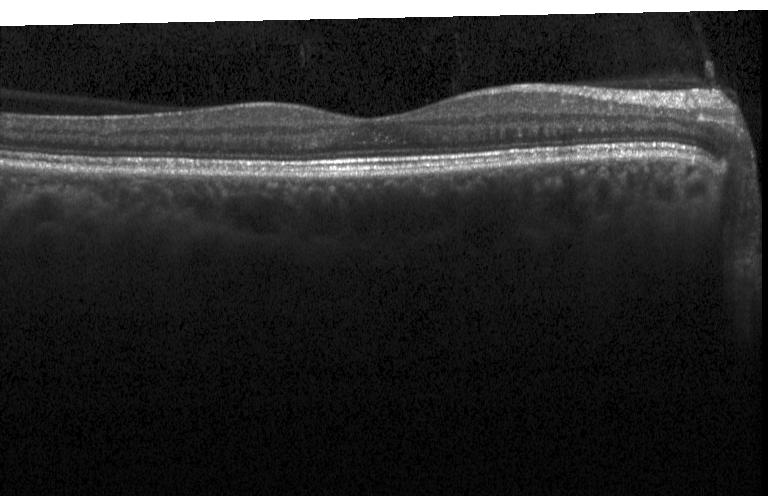 The scan shows no CNV, no DME, and no drusen.